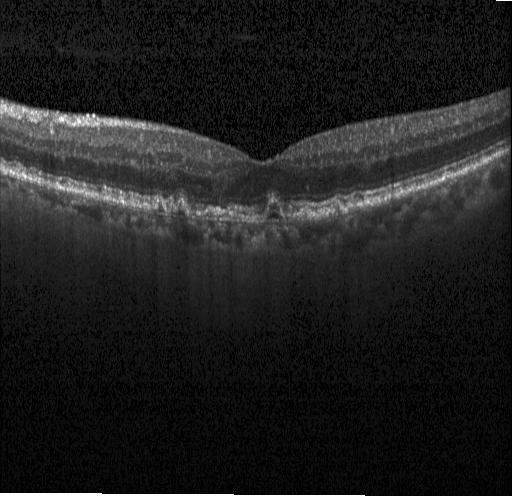
Retinal OCT B-scan
Macular OCT: multiple drusen.